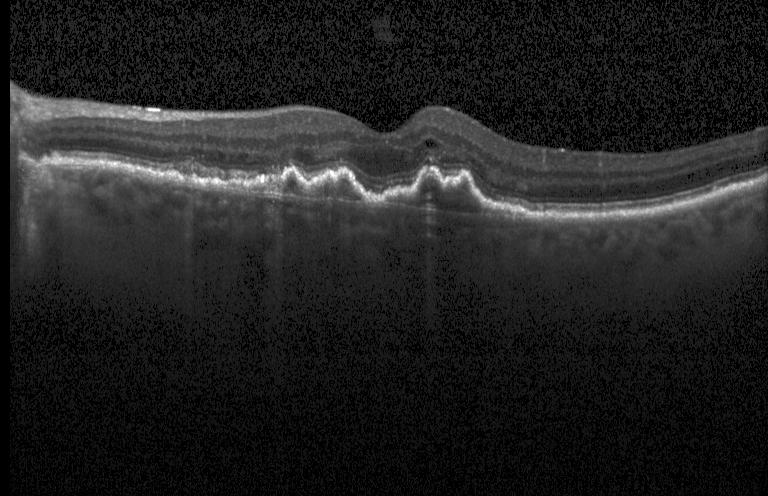

Optical coherence tomography scan; Heidelberg Spectralis; spectral-domain optical coherence tomography
Diagnosis: a choroidal neovascular membrane.